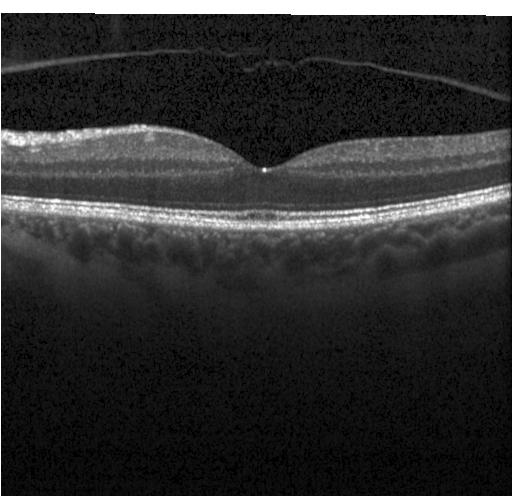

Spectral-domain OCT. Fovea-centered. Instrument: Heidelberg Spectralis. OCT line scan
Impression: no choroidal neovascularization, diabetic macular edema, or drusen.